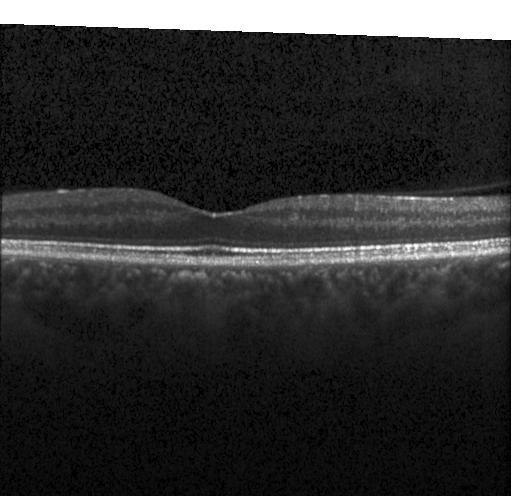 Spectral-domain optical coherence tomography · macular scan · OCT line scan · Heidelberg Spectralis OCT system.
Assessment: neither choroidal neovascularization, diabetic macular edema, nor drusen.